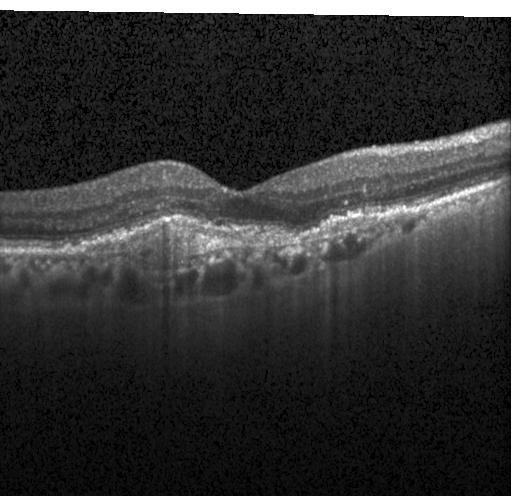 Spectral-domain OCT B-scan: a choroidal neovascular membrane.